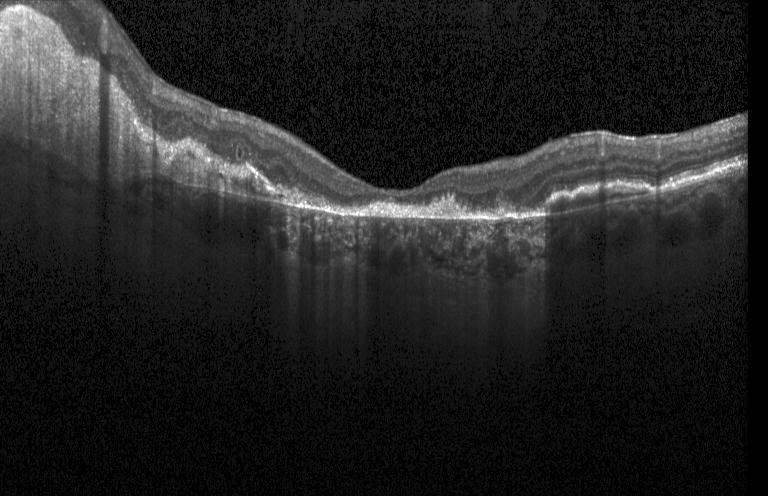
OCT B-scan.
Finding: a choroidal neovascular membrane.